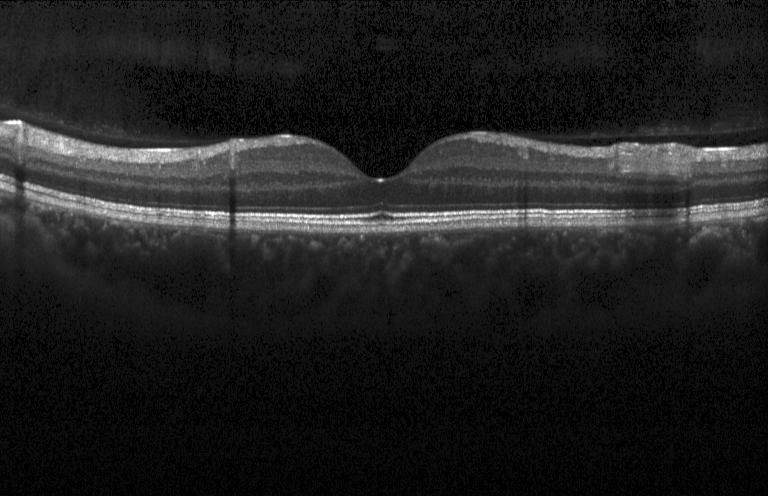 OCT line scan. Horizontal scan through the fovea. Heidelberg Spectralis — Dx: no choroidal neovascularization, no diabetic macular edema, and no drusen.